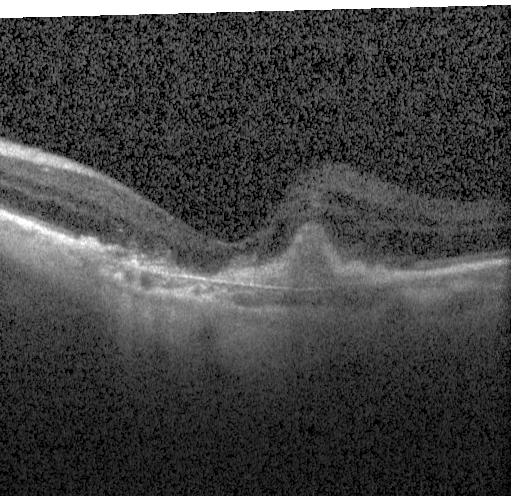 Retinal OCT B-scan. Assessment: choroidal neovascularization.